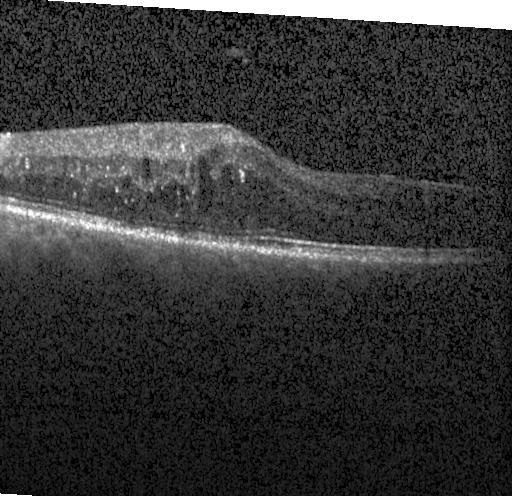
Retinal OCT B-scan · Heidelberg Spectralis OCT system — Finding: DME.